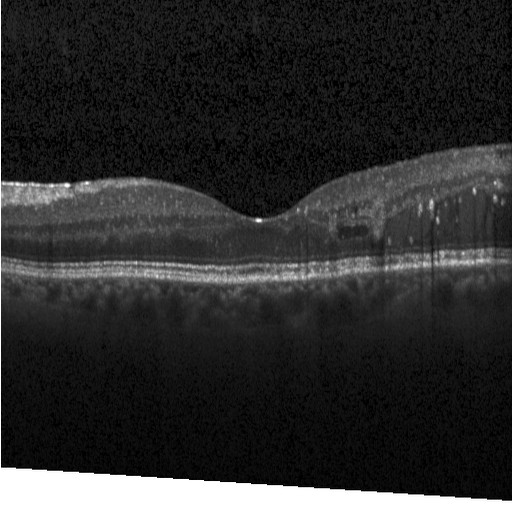

Optical coherence tomography scan, fovea-centered
Assessment: diabetic macular edema (DME).